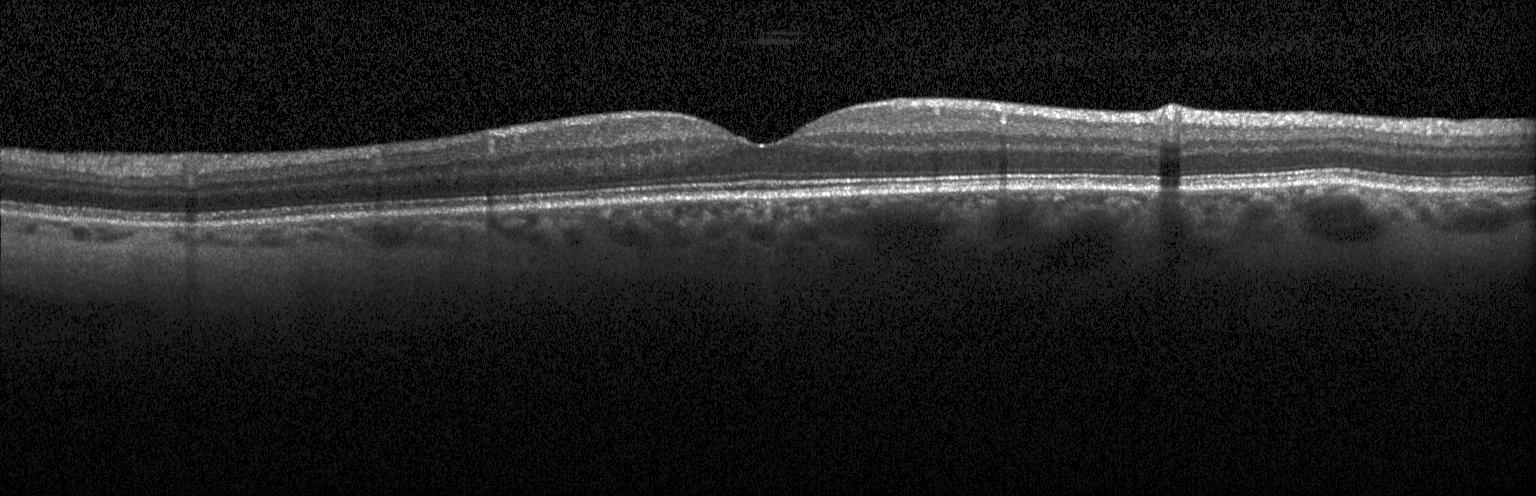 Spectral-domain OCT, through the macula, Heidelberg Spectralis, OCT line scan.
Finding: neither CNV, DME, nor drusen.